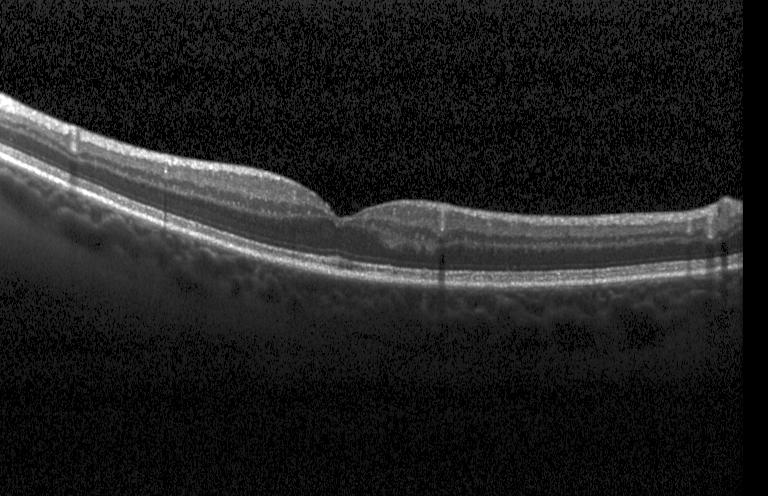 OCT finding: neither choroidal neovascularization, diabetic macular edema, nor drusen.